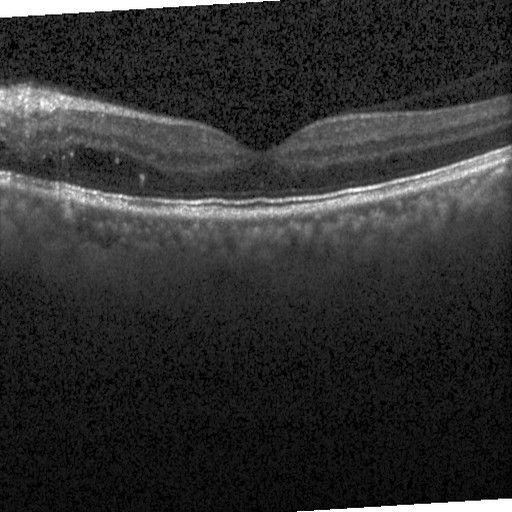
Finding: diabetic macular edema.